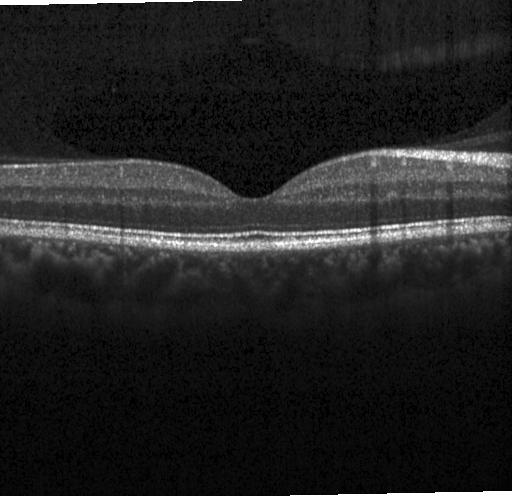

Finding: no choroidal neovascularization, diabetic macular edema, or drusen.